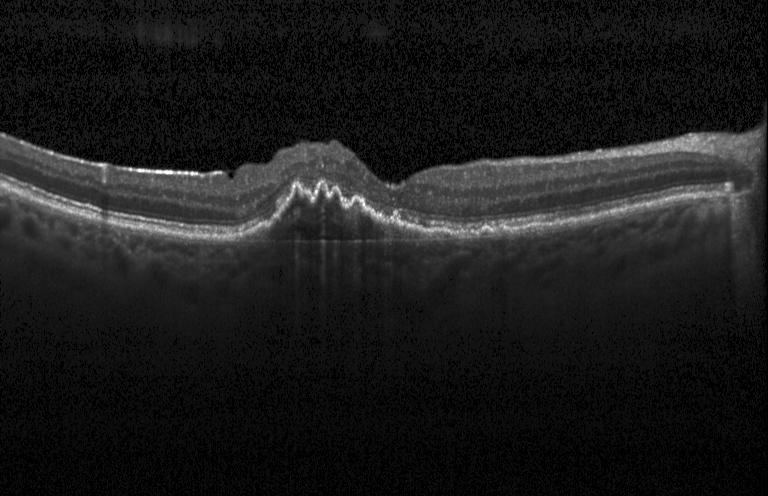 Optical coherence tomography scan; Heidelberg Spectralis; fovea-centered; spectral-domain OCT.
Dx: choroidal neovascularization (CNV).